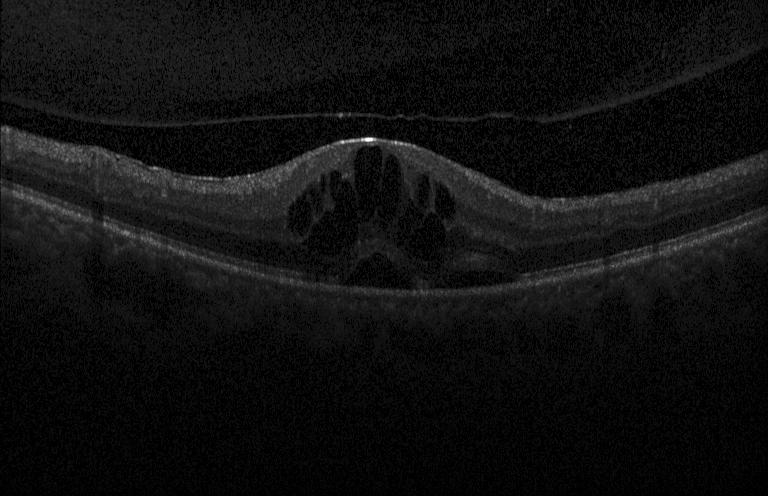

Heidelberg Spectralis OCT system. SD-OCT. Retinal OCT B-scan. Macular scan. DME.